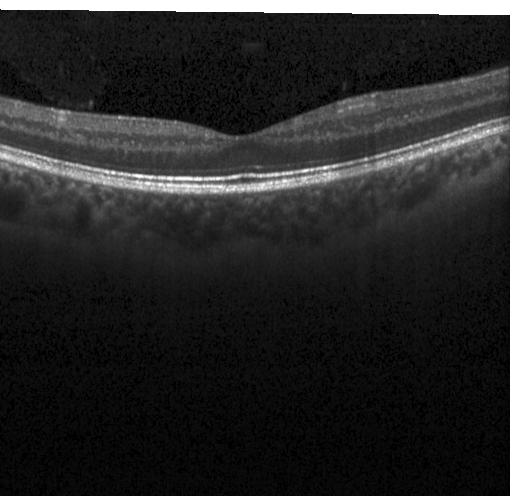
OCT line scan
Impression: neither choroidal neovascularization, diabetic macular edema, nor drusen.